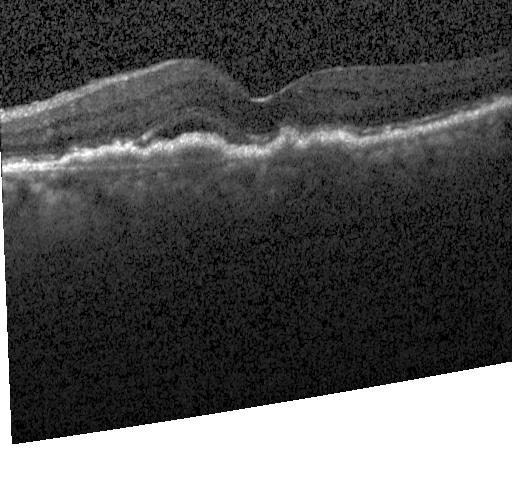

Instrument: Heidelberg Spectralis, retinal OCT cross-section, through the macula — OCT finding: CNV.